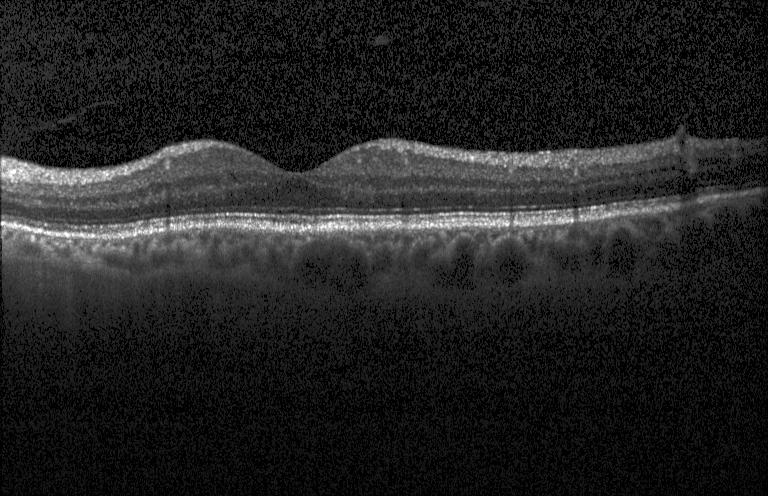 Horizontal scan through the fovea. Spectral-domain optical coherence tomography. Retinal OCT cross-section
OCT finding: neither choroidal neovascularization, diabetic macular edema, nor drusen.